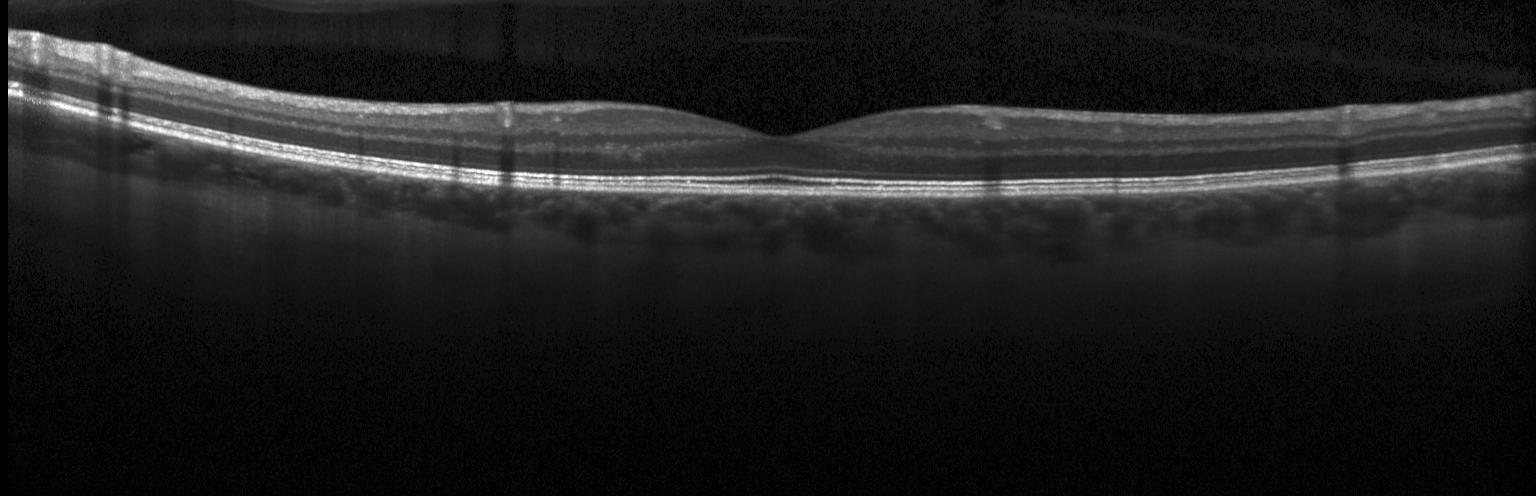

Macular scan · Heidelberg Spectralis · retinal OCT B-scan · spectral-domain optical coherence tomography.
The scan shows no CNV, DME, or drusen.